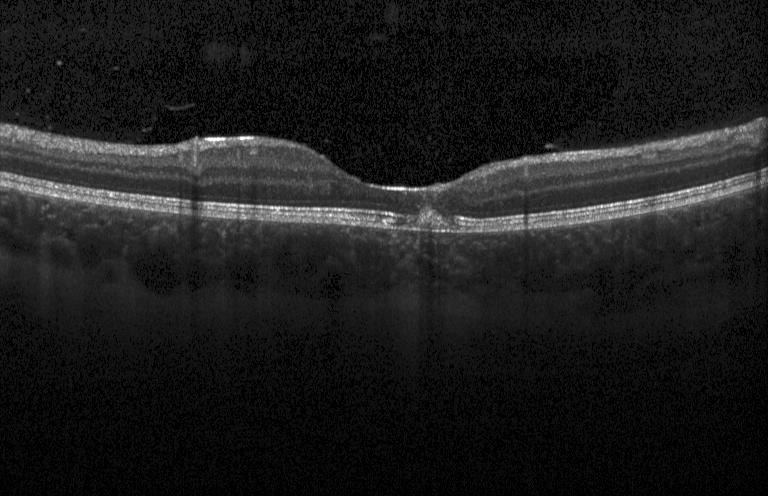

Macular scan; spectral-domain optical coherence tomography; OCT line scan; Heidelberg Spectralis OCT system.
Assessment: CNV.